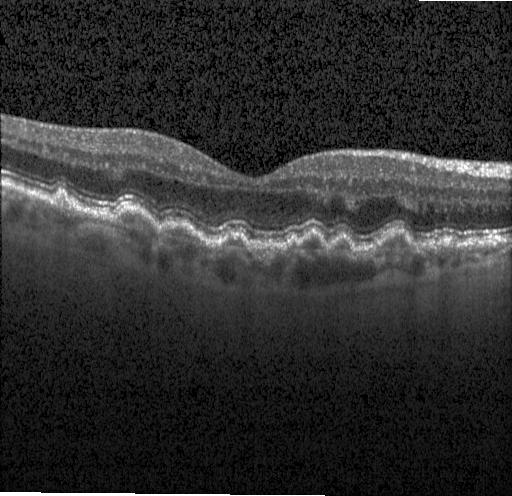

Macular OCT: drusen.